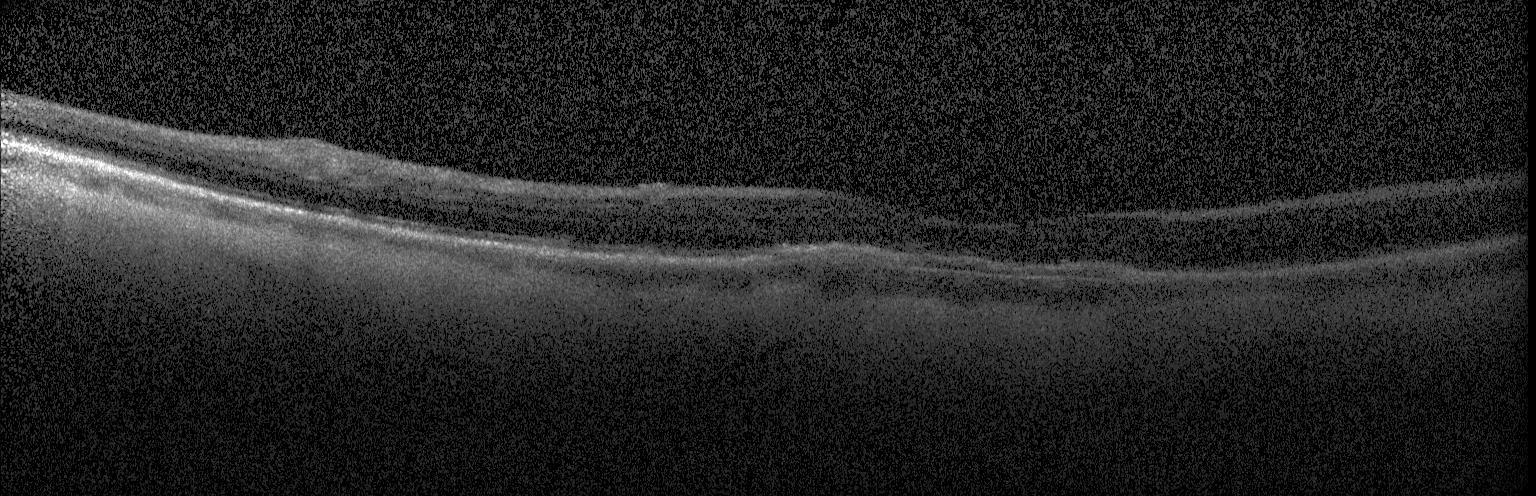
Instrument: Heidelberg Spectralis, through the macula, retinal OCT B-scan, spectral-domain OCT
Finding: choroidal neovascularization (CNV).